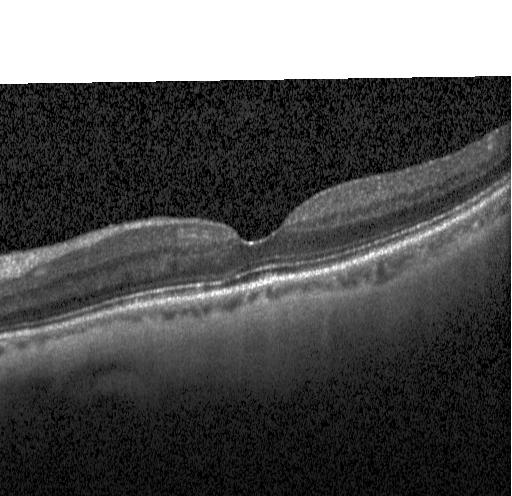 Spectral-domain optical coherence tomography. Centered on the fovea. Retinal OCT cross-section — OCT finding: no evidence of choroidal neovascularization, diabetic macular edema, or drusen.